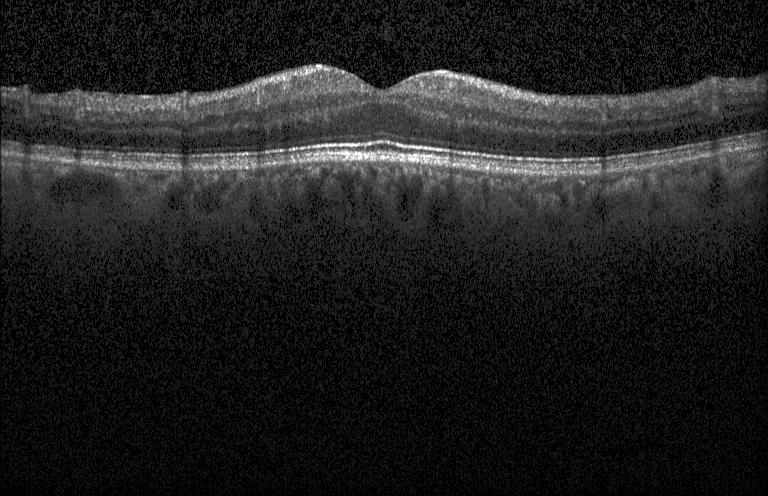 Impression: neither CNV, DME, nor drusen.